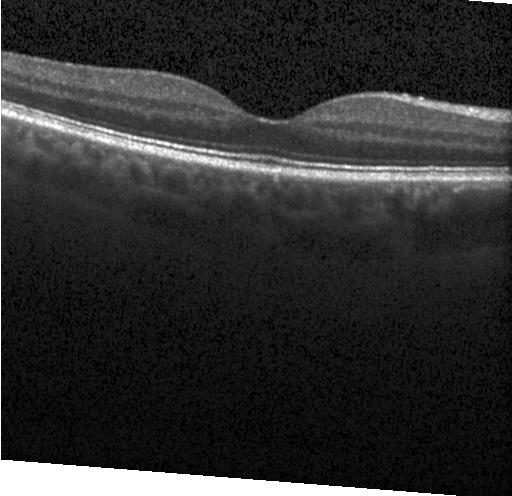 Retinal OCT cross-section
Diagnosis: neither choroidal neovascularization, diabetic macular edema, nor drusen.